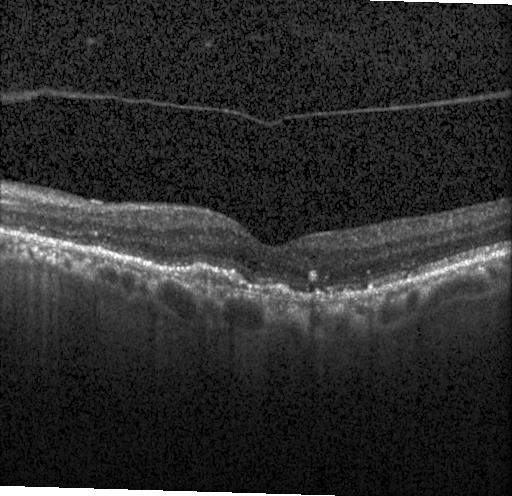 OCT B-scan showing choroidal neovascularization (CNV).